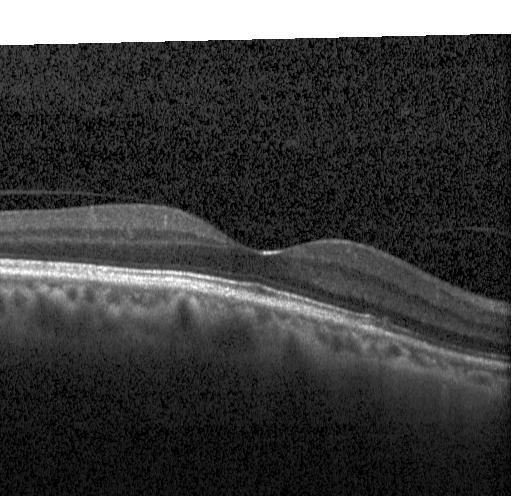 OCT scan showing no evidence of choroidal neovascularization, diabetic macular edema, or drusen.